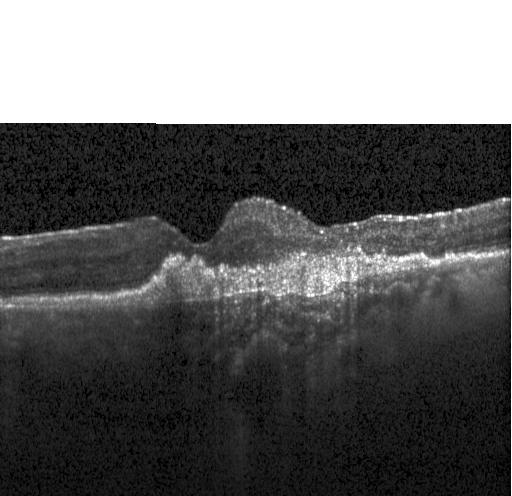

Spectral-domain OCT; acquired on a Heidelberg Spectralis; fovea-centered; optical coherence tomography scan.
OCT finding: choroidal neovascularization (CNV).